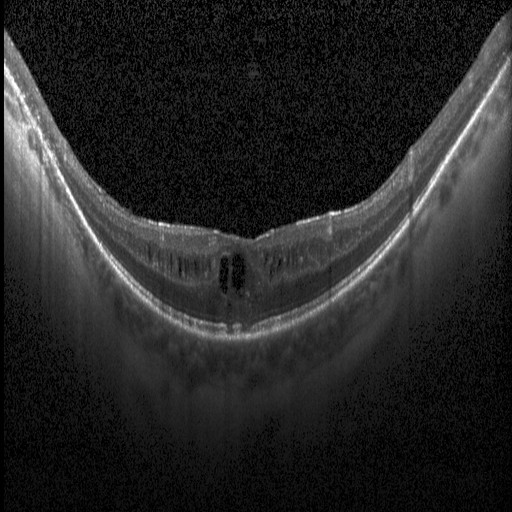
OCT B-scan, Heidelberg Spectralis OCT system, horizontal scan through the fovea, spectral-domain OCT — Assessment: diabetic macular edema (DME).